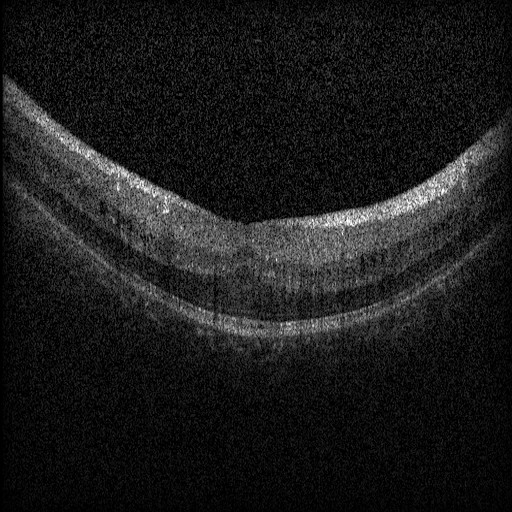

Diabetic macular edema.